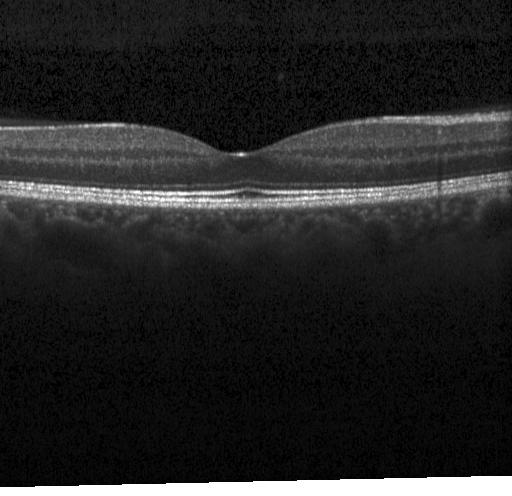 Finding: no evidence of choroidal neovascularization, diabetic macular edema, or drusen.